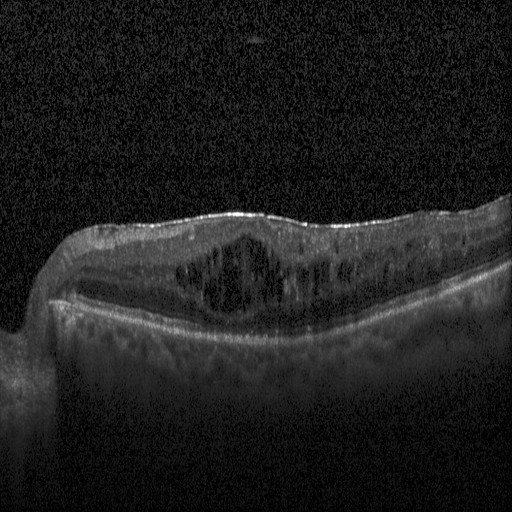 SD-OCT. Retinal OCT B-scan — Assessment: diabetic macular edema.